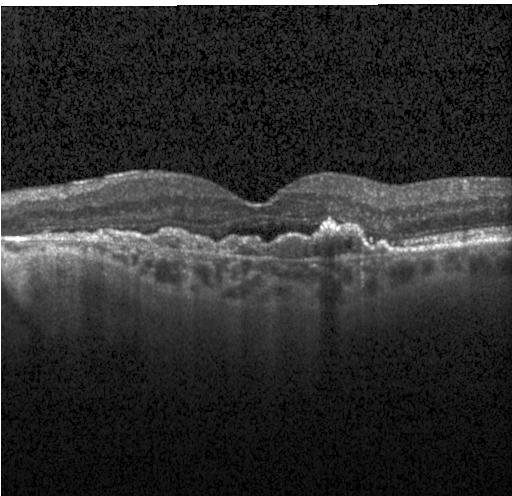 OCT line scan. Horizontal scan through the fovea. SD-OCT. Finding: a choroidal neovascular membrane.